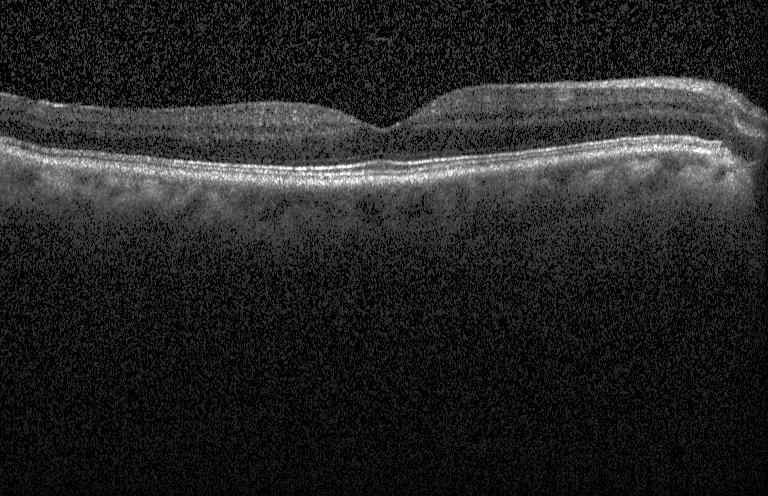

Spectral-domain optical coherence tomography. Macular scan. Retinal OCT cross-section. Acquired on a Heidelberg Spectralis.
Finding: no choroidal neovascularization, no diabetic macular edema, and no drusen.